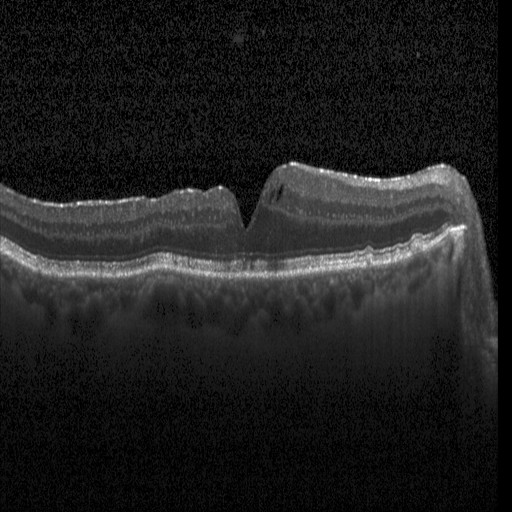

OCT B-scan, macular scan — Finding: diabetic macular edema (DME).